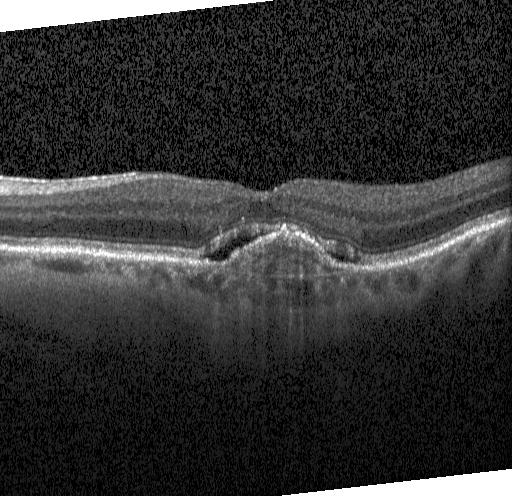
Impression: choroidal neovascularization (CNV).